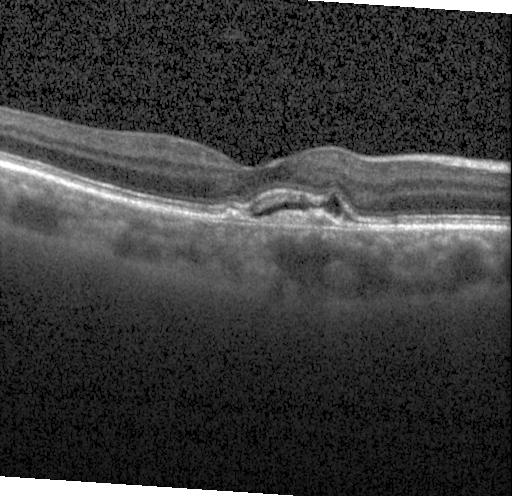 SD-OCT; centered on the fovea; OCT line scan; acquired on a Heidelberg Spectralis. Finding: choroidal neovascularization.